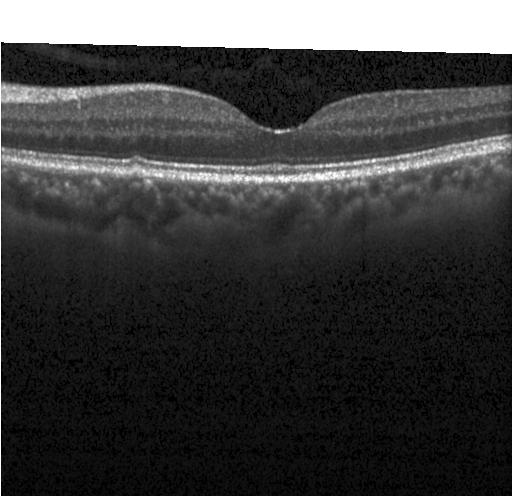
Optical coherence tomography B-scan.
The scan shows multiple drusen.